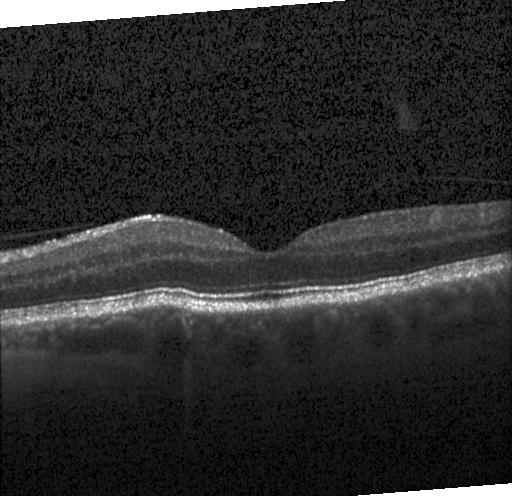

Heidelberg Spectralis OCT system; macular scan; OCT B-scan; spectral-domain optical coherence tomography. The scan shows neither choroidal neovascularization, diabetic macular edema, nor drusen.